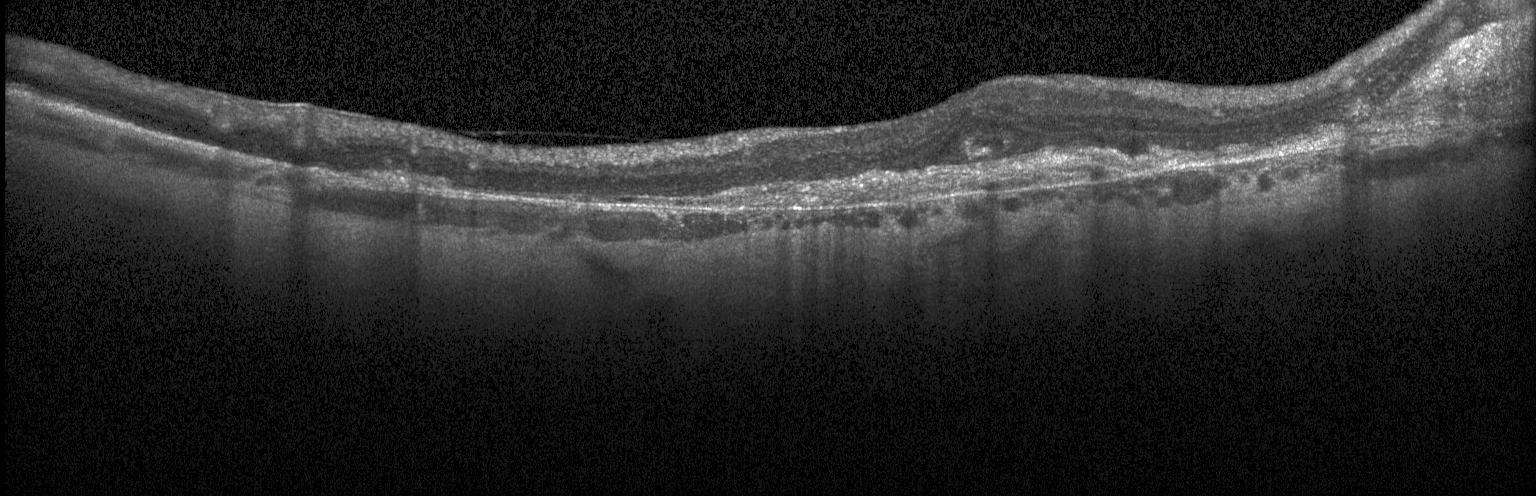
Retinal OCT cross-section showing a choroidal neovascular membrane.